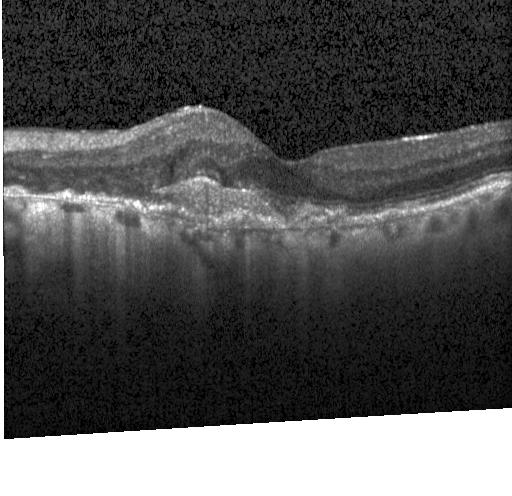
Dx: CNV.